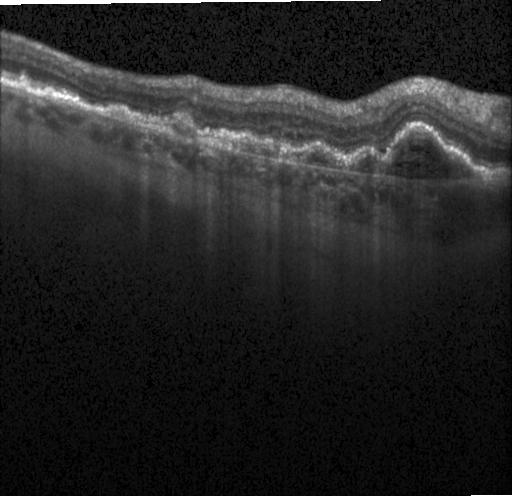 Optical coherence tomography B-scan · Heidelberg Spectralis OCT system · spectral-domain optical coherence tomography · centered on the fovea — Assessment: a choroidal neovascular membrane.